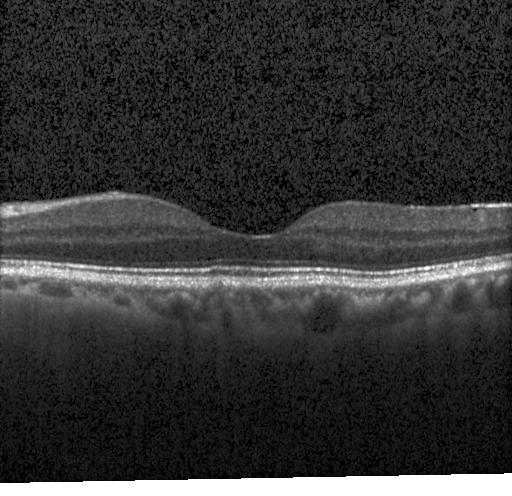
OCT B-scan. Heidelberg Spectralis OCT system.
Impression: neither CNV, DME, nor drusen.